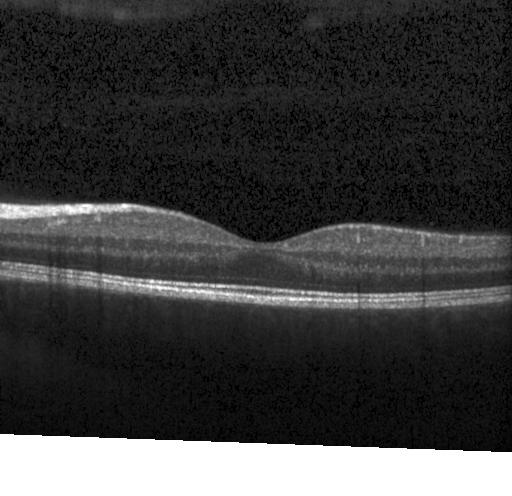
OCT B-scan · spectral-domain OCT · fovea-centered — Dx: no evidence of choroidal neovascularization, diabetic macular edema, or drusen.